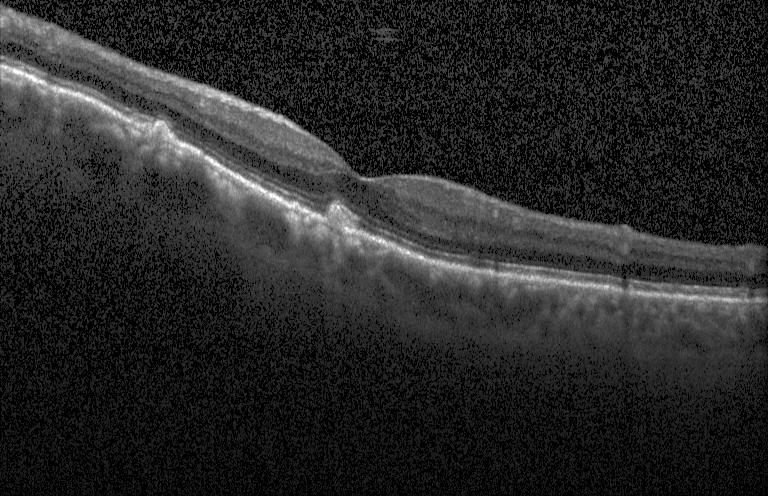

Diagnosis: drusen.